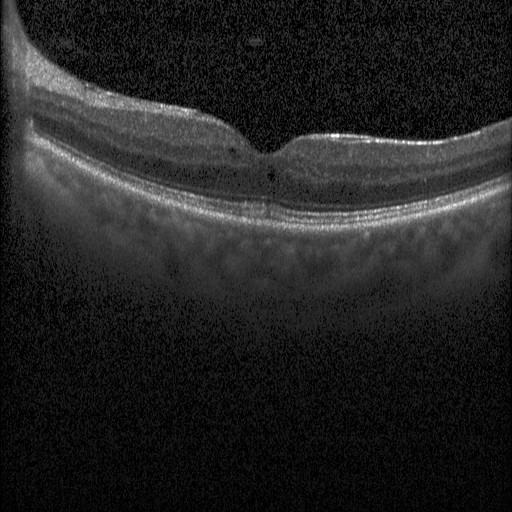 Retinal OCT B-scan. SD-OCT.
Impression: DME.